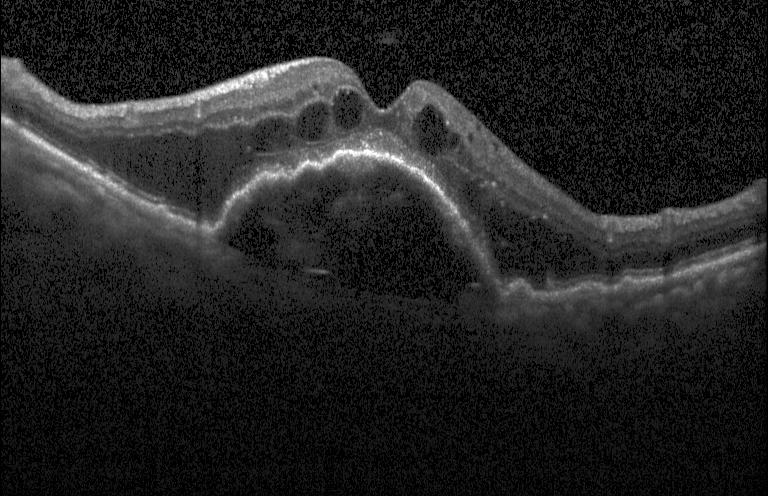

OCT scan showing choroidal neovascularization.